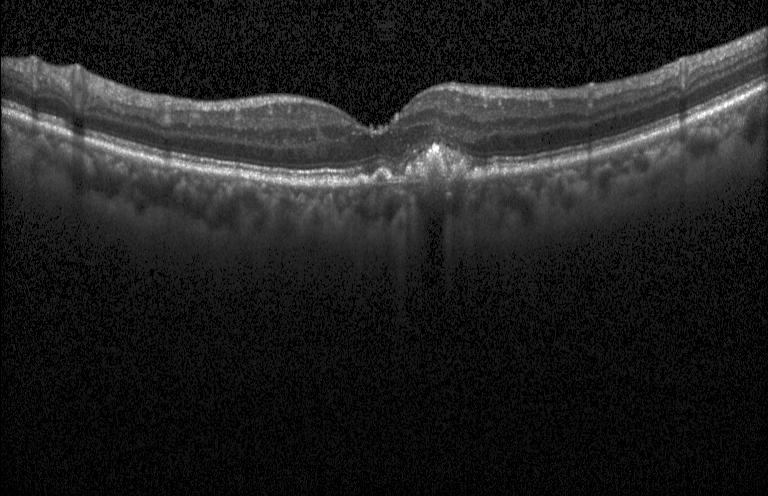

Heidelberg Spectralis, optical coherence tomography B-scan
Assessment: multiple drusen.